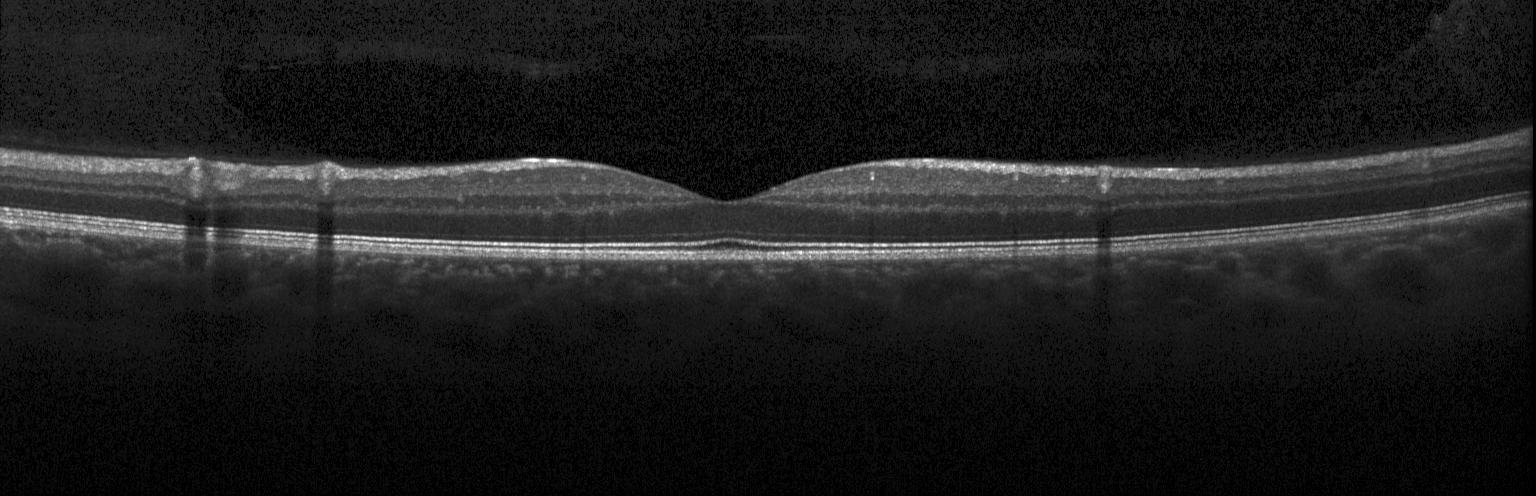 Spectral-domain OCT B-scan: neither choroidal neovascularization, diabetic macular edema, nor drusen.